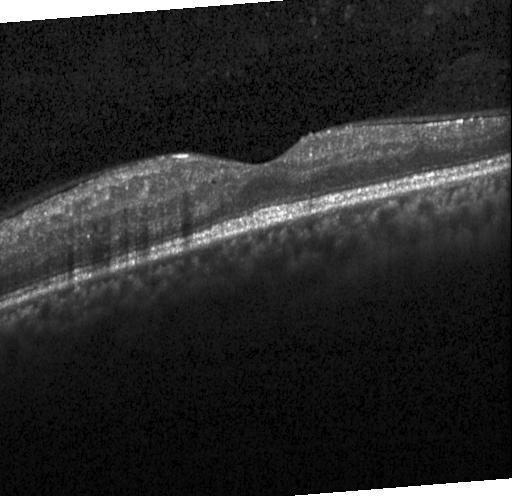
OCT line scan — Finding: diabetic macular edema.